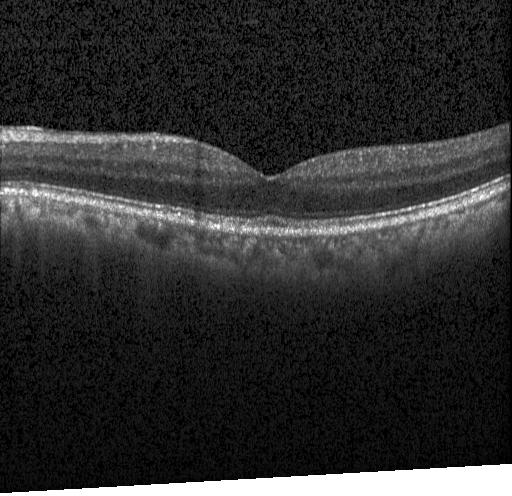
Dx: no CNV, DME, or drusen.